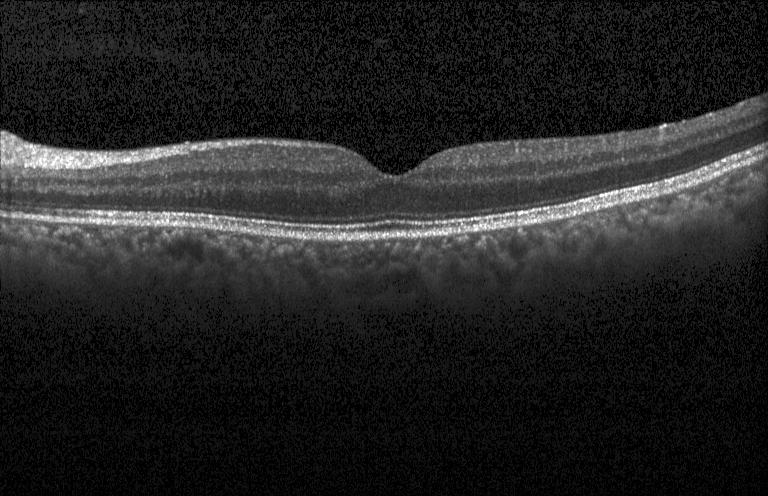 The scan shows no choroidal neovascularization, no diabetic macular edema, and no drusen.